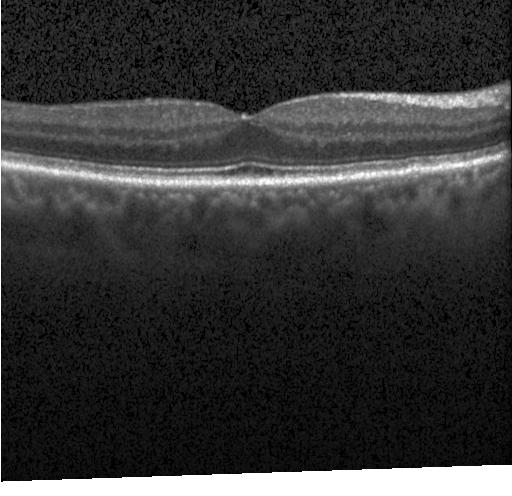 Assessment: no CNV, no DME, and no drusen.